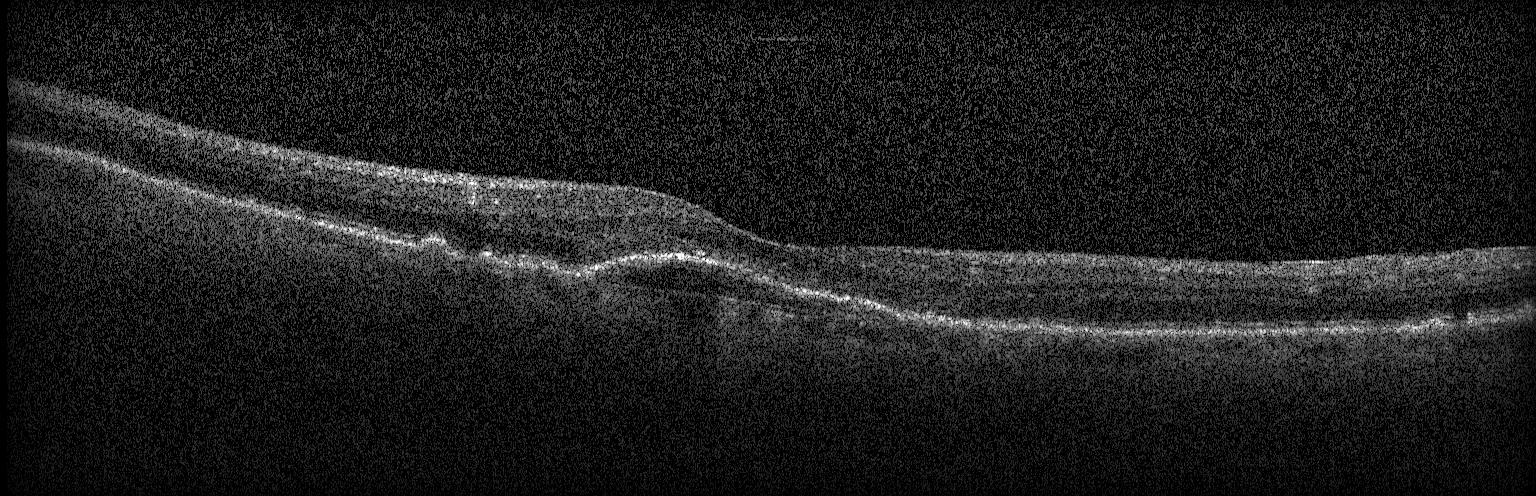 Spectral-domain optical coherence tomography. Instrument: Heidelberg Spectralis. Optical coherence tomography scan
Impression: choroidal neovascularization.